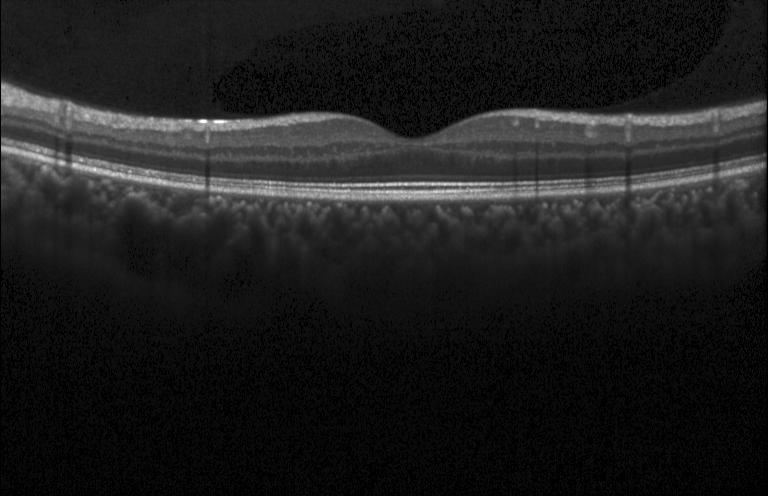

Spectral-domain optical coherence tomography, retinal OCT cross-section
Impression: no choroidal neovascularization, no diabetic macular edema, and no drusen.